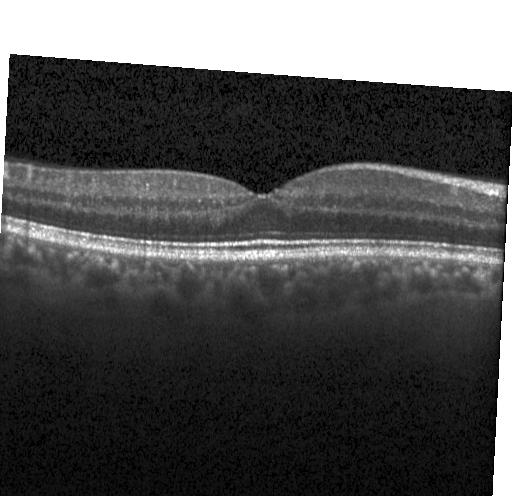

The scan shows no evidence of choroidal neovascularization, diabetic macular edema, or drusen.